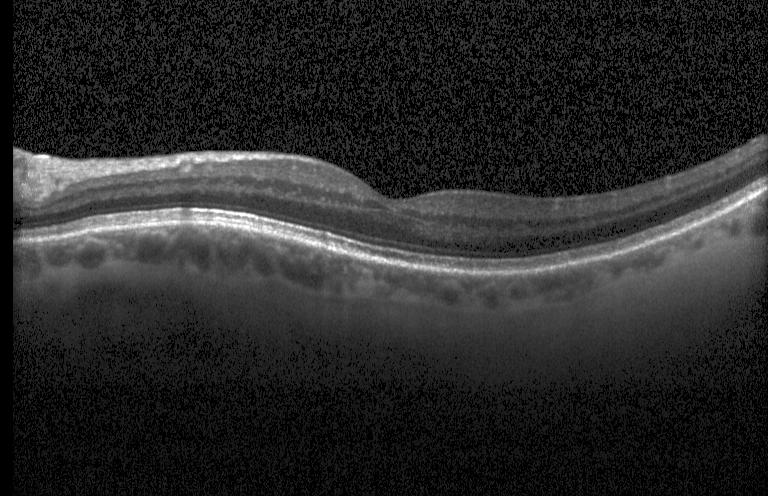

Optical coherence tomography B-scan; macular scan.
The scan shows no evidence of choroidal neovascularization, diabetic macular edema, or drusen.